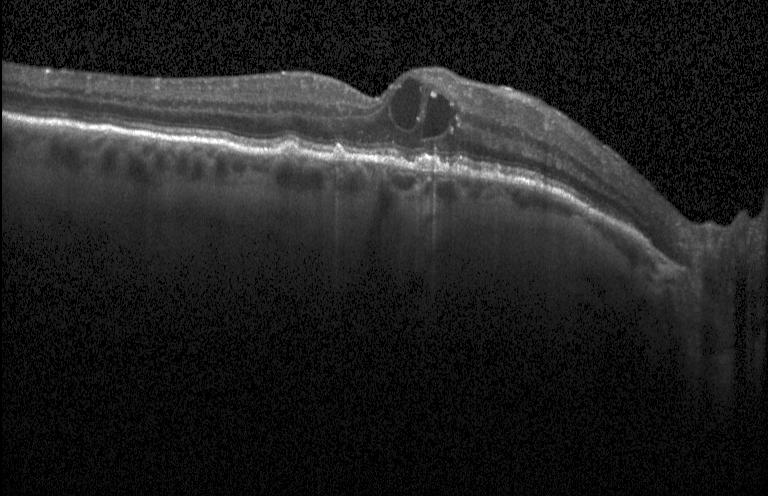
Centered on the fovea · OCT B-scan.
Assessment: a choroidal neovascular membrane.